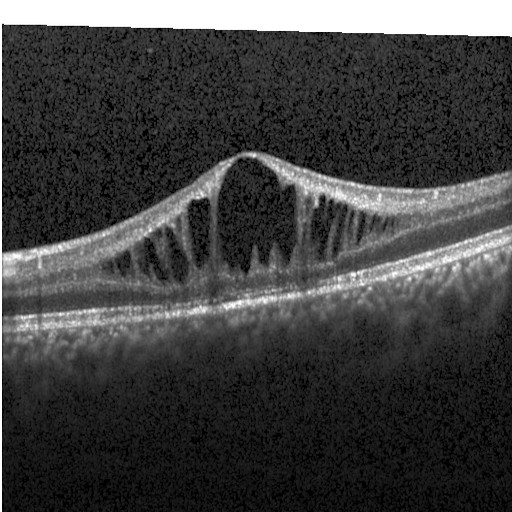
Acquired on a Heidelberg Spectralis. Optical coherence tomography B-scan.
This B-scan demonstrates diabetic macular edema.